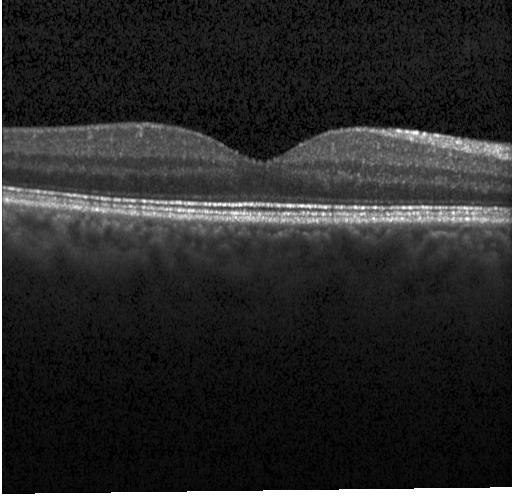

Assessment: no evidence of choroidal neovascularization, diabetic macular edema, or drusen.